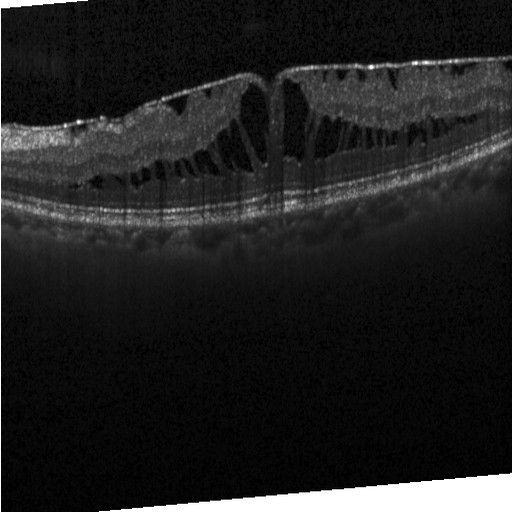

OCT B-scan · instrument: Heidelberg Spectralis · fovea-centered
Finding: diabetic macular edema.